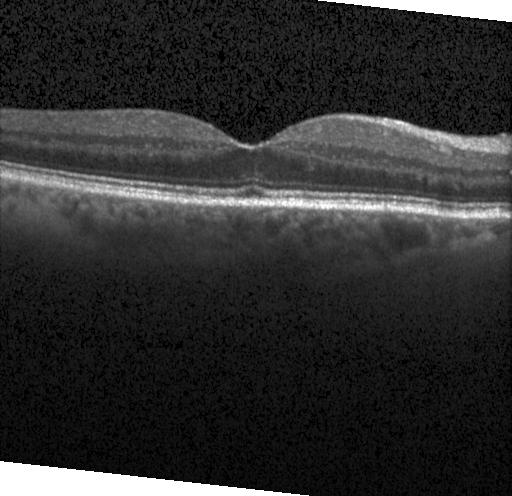
Optical coherence tomography scan, spectral-domain OCT.
Diagnosis: neither choroidal neovascularization, diabetic macular edema, nor drusen.